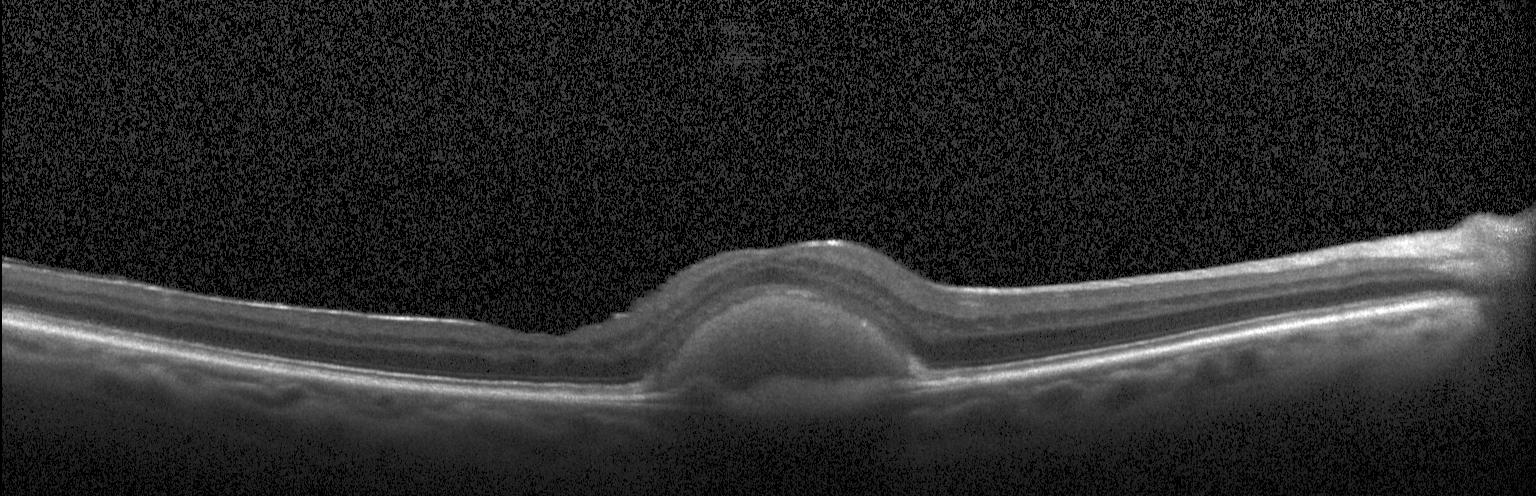 Horizontal scan through the fovea; SD-OCT; optical coherence tomography scan — Finding: choroidal neovascularization.